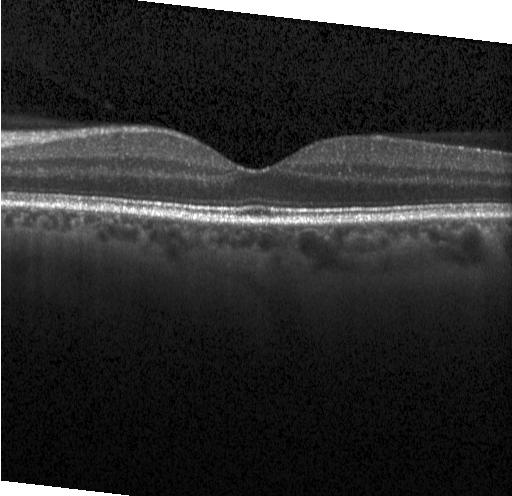 Spectral-domain OCT, fovea-centered, OCT line scan — Dx: no choroidal neovascularization, no diabetic macular edema, and no drusen.